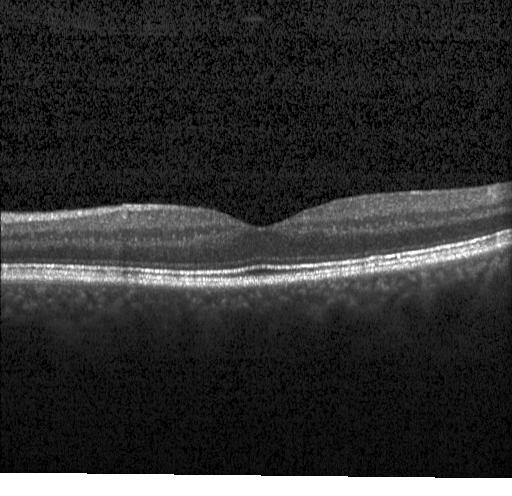 Heidelberg Spectralis OCT system; macular scan; SD-OCT; optical coherence tomography B-scan — Diagnosis: no choroidal neovascularization, no diabetic macular edema, and no drusen.